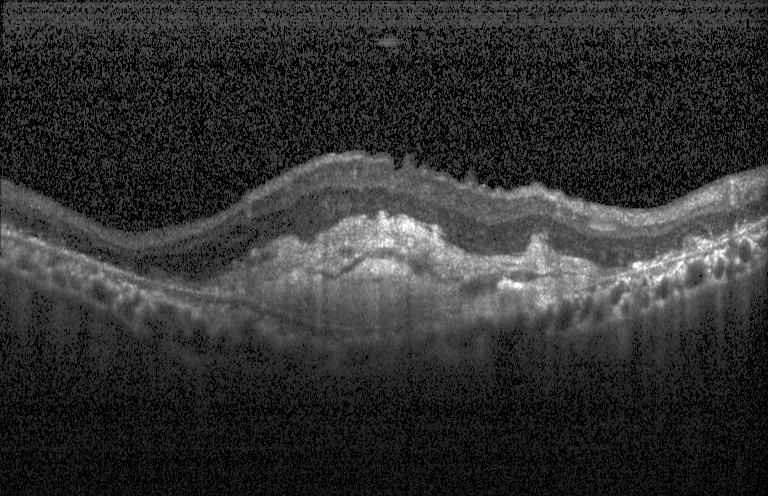
Instrument: Heidelberg Spectralis, through the macula, retinal OCT cross-section. Finding: choroidal neovascularization (CNV).